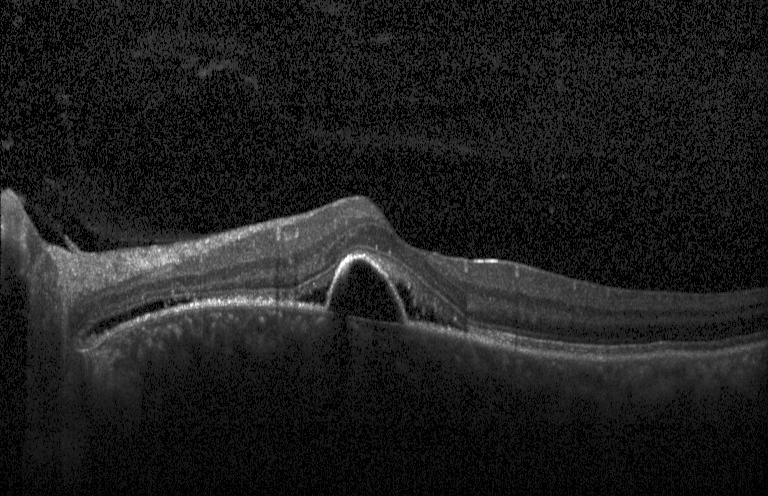

This B-scan demonstrates a choroidal neovascular membrane.